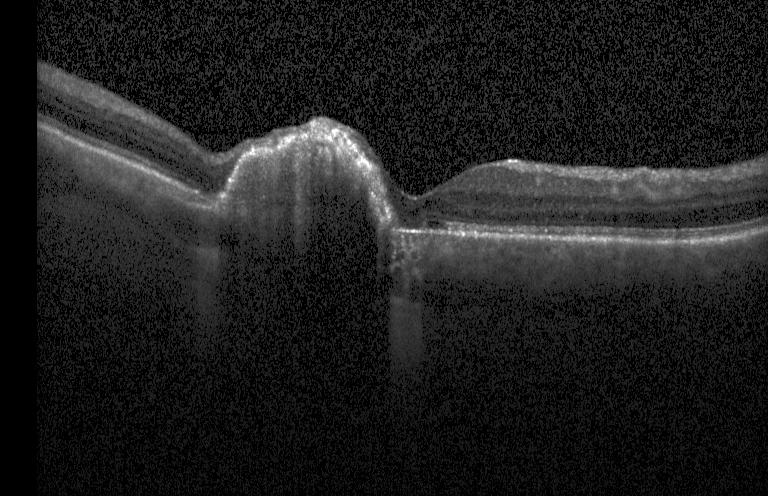
This B-scan demonstrates a choroidal neovascular membrane.